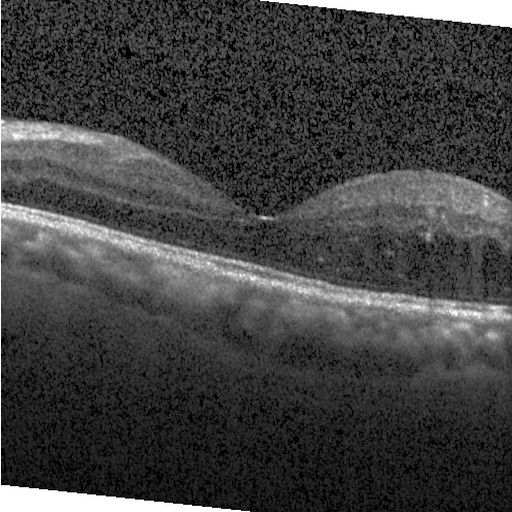
Retinal OCT B-scan. Instrument: Heidelberg Spectralis. Spectral-domain OCT
Macular OCT: diabetic macular edema (DME).